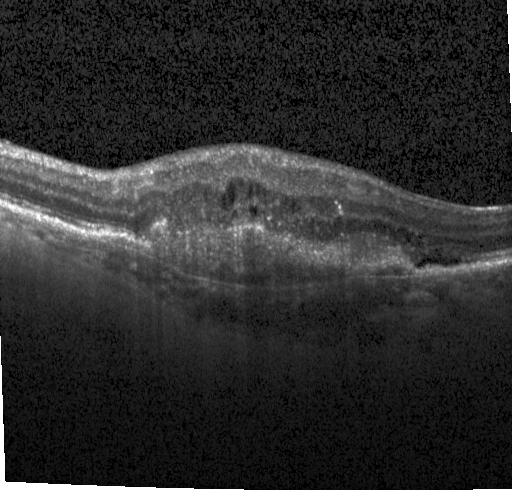

Diagnosis: CNV.